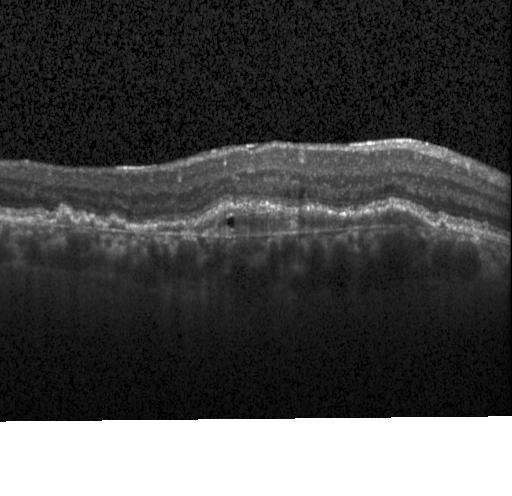
Dx: a choroidal neovascular membrane.